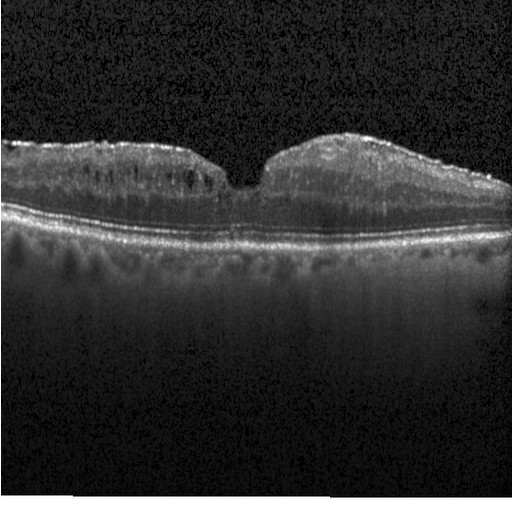 Retinal OCT cross-section showing diabetic macular edema (DME).